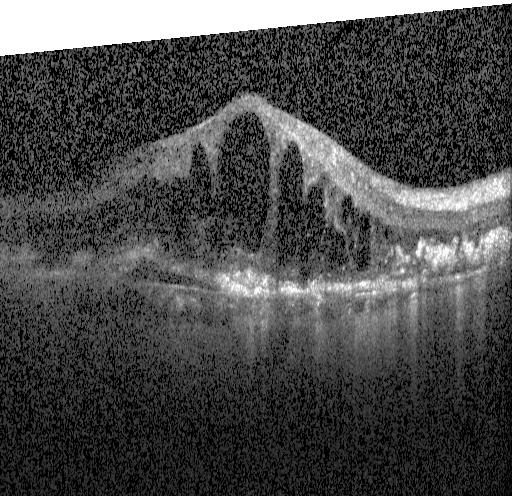 Retinal OCT cross-section showing CNV.